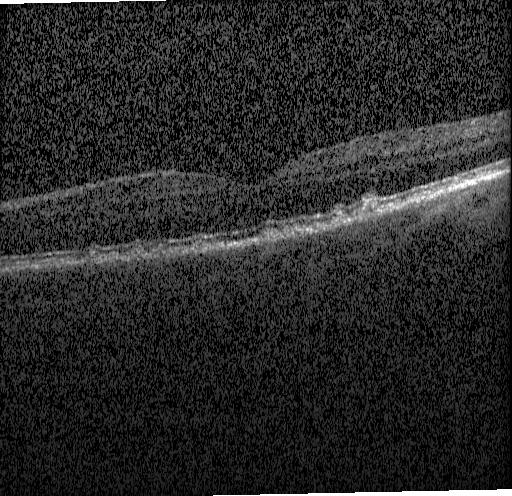

OCT B-scan — The scan shows drusen.